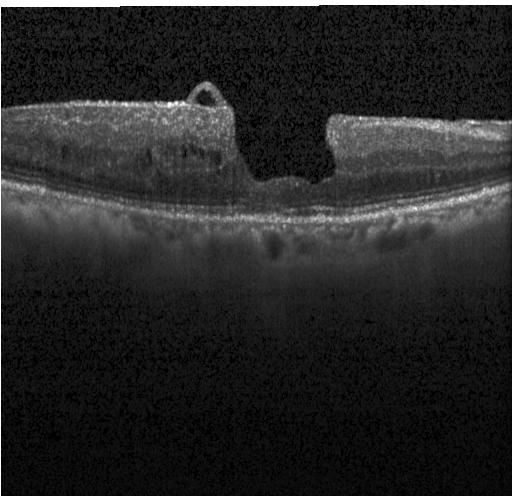

The scan shows DME.